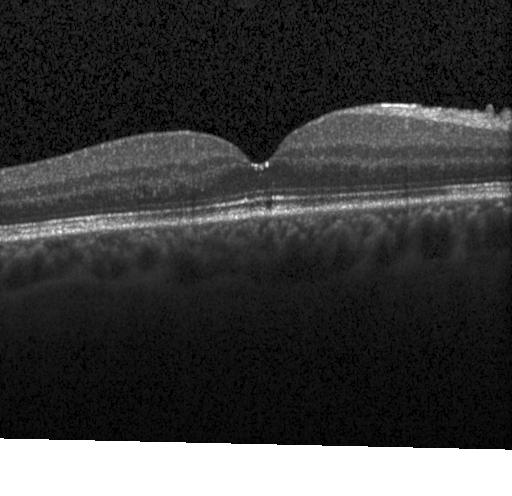 Optical coherence tomography B-scan. Through the macula. SD-OCT. Heidelberg Spectralis OCT system. OCT finding: no choroidal neovascularization, diabetic macular edema, or drusen.